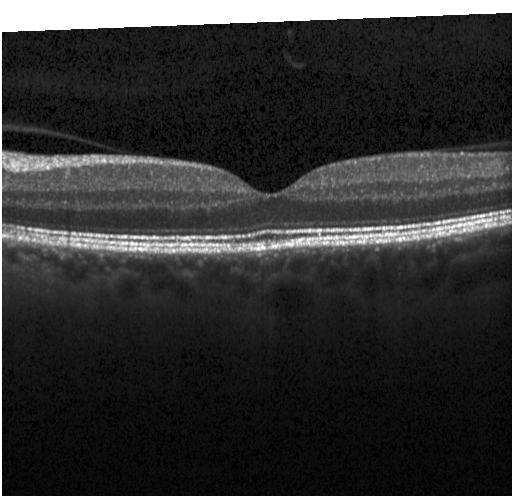 OCT line scan. Heidelberg Spectralis OCT system. Centered on the fovea — Diagnosis: no evidence of choroidal neovascularization, diabetic macular edema, or drusen.